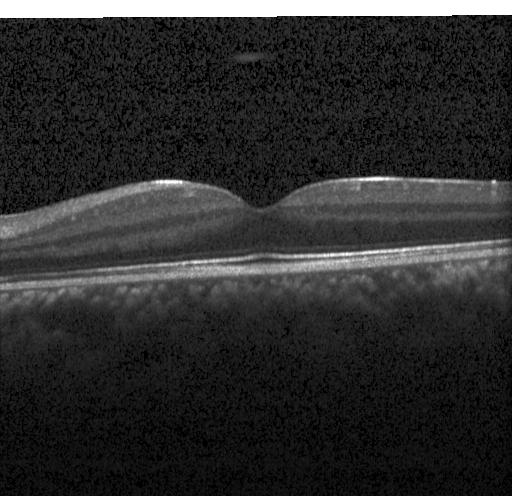

Diagnosis: no choroidal neovascularization, no diabetic macular edema, and no drusen.